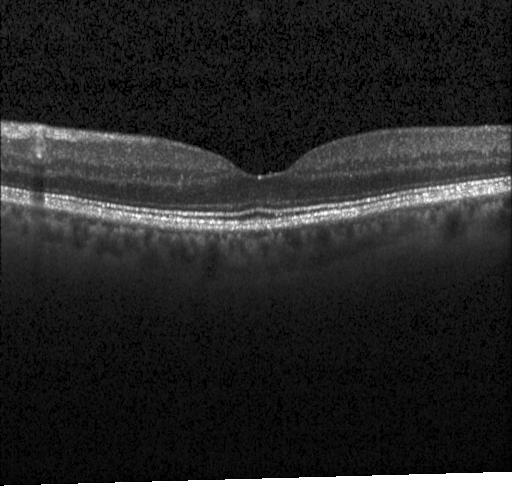
Centered on the fovea. Optical coherence tomography scan. Macular OCT: no choroidal neovascularization, diabetic macular edema, or drusen.